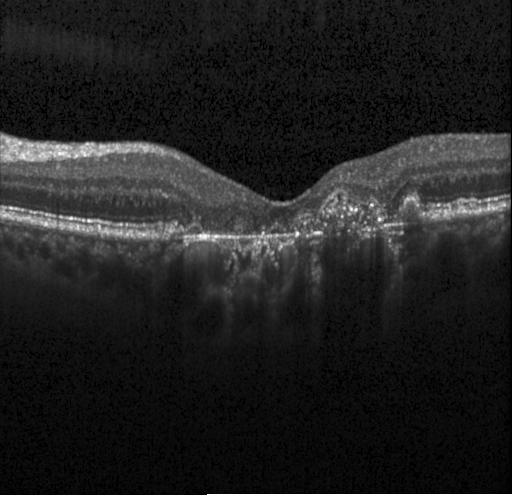

Macular OCT demonstrating a choroidal neovascular membrane.